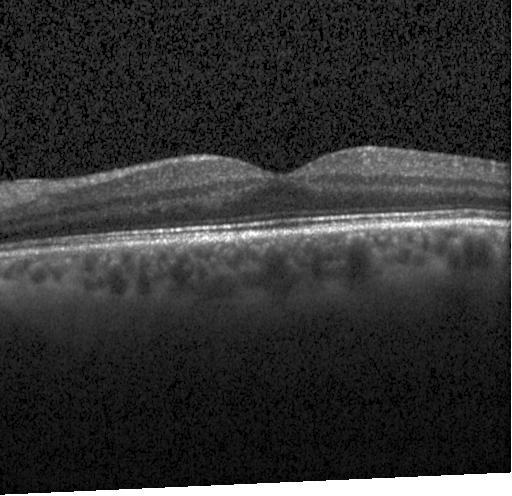

Optical coherence tomography B-scan — Finding: no choroidal neovascularization, diabetic macular edema, or drusen.